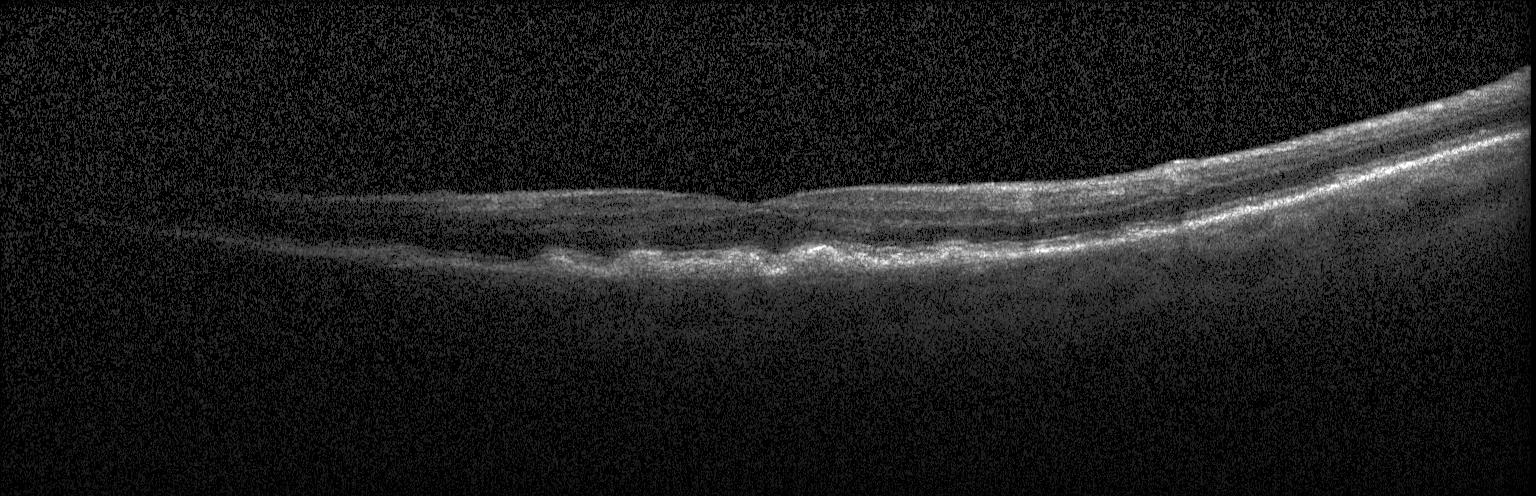 Horizontal scan through the fovea · optical coherence tomography B-scan · spectral-domain OCT · Heidelberg Spectralis.
Multiple drusen.